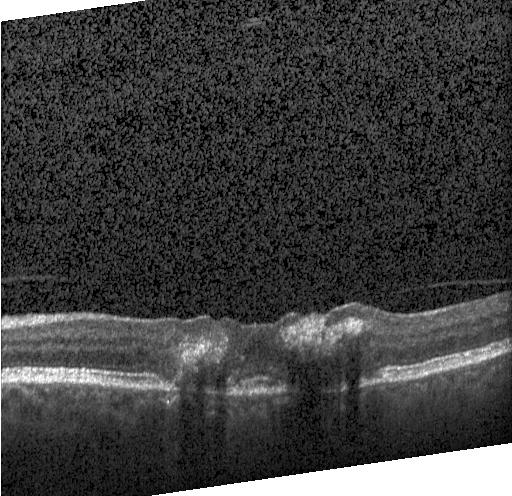 Heidelberg Spectralis OCT system, spectral-domain OCT, retinal OCT B-scan, through the macula
Dx: a choroidal neovascular membrane.